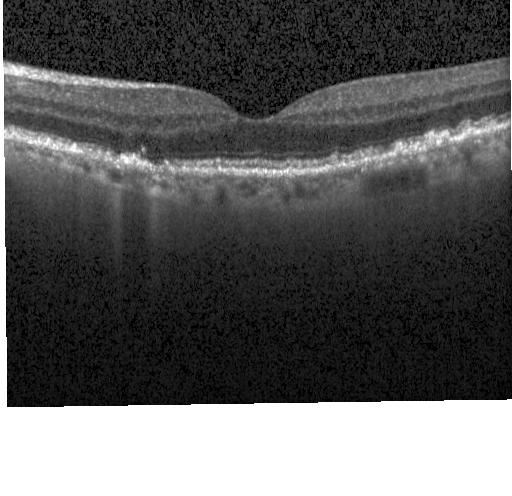

Heidelberg Spectralis · horizontal scan through the fovea · optical coherence tomography scan. Finding: multiple drusen.